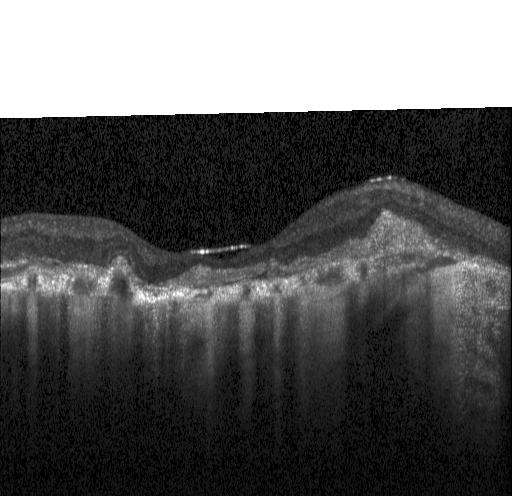
Centered on the fovea. Instrument: Heidelberg Spectralis. Optical coherence tomography B-scan — Assessment: choroidal neovascularization.